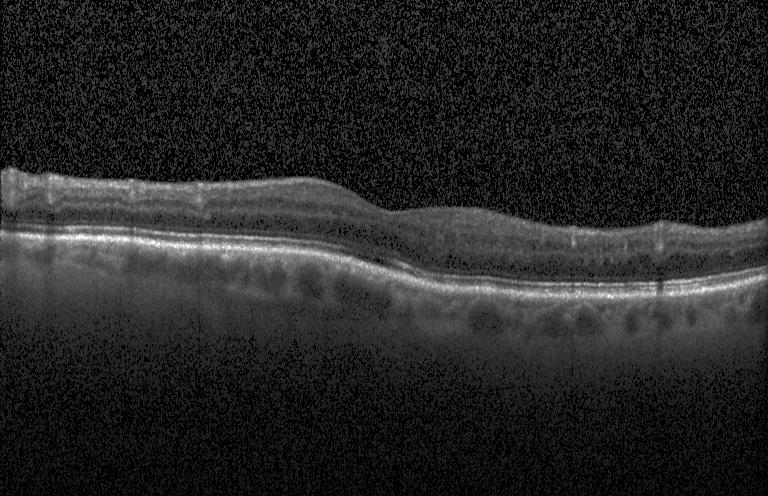 Dx: no CNV, DME, or drusen.